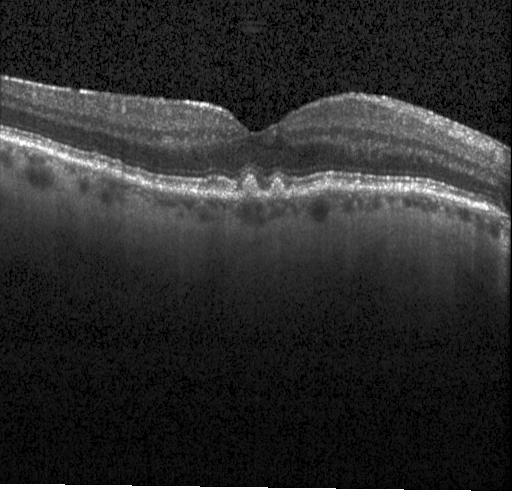
Diagnosis: multiple drusen.